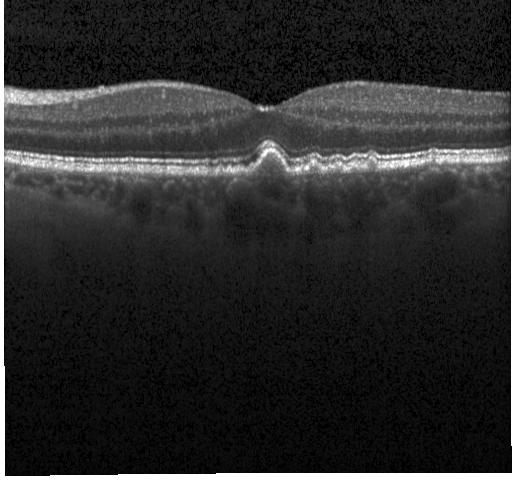

Finding: drusen.